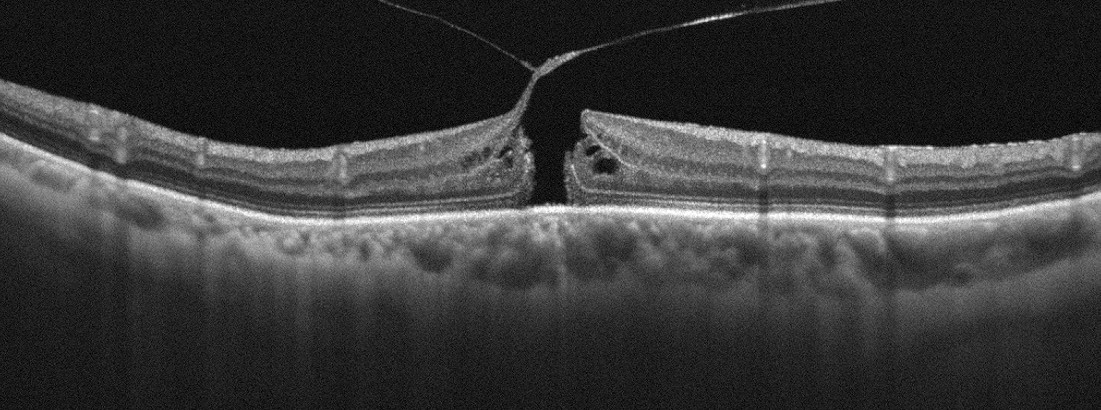

OCT line scan. Assessment: vitreomacular interface disease.